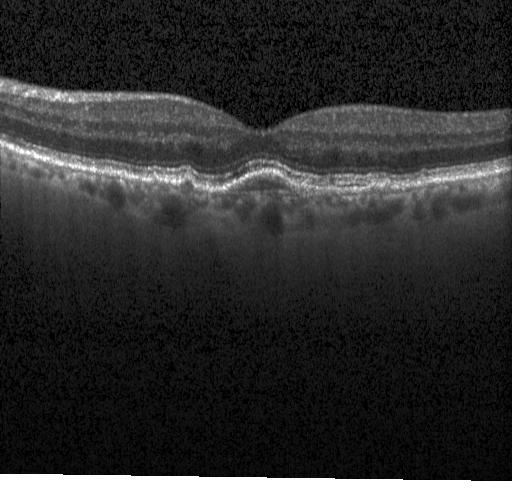 The scan shows CNV.